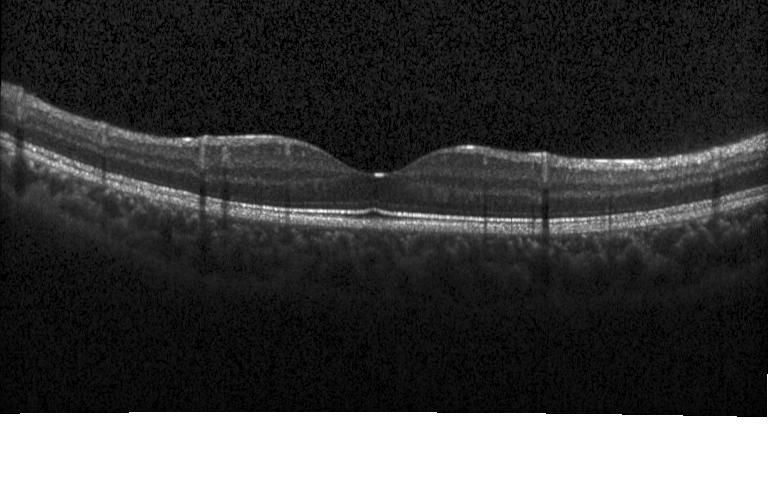 Retinal OCT cross-section. No evidence of choroidal neovascularization, diabetic macular edema, or drusen.